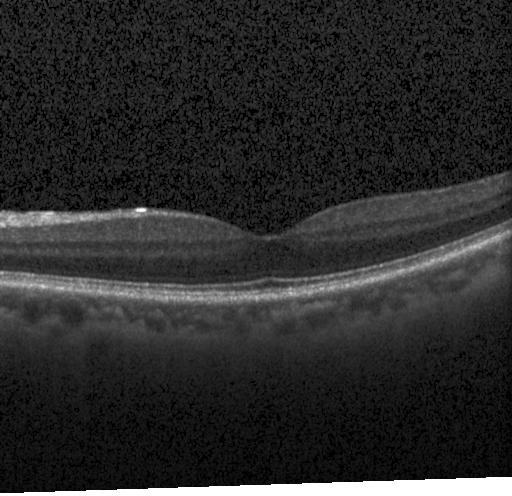 Optical coherence tomography scan; instrument: Heidelberg Spectralis
Finding: no CNV, no DME, and no drusen.